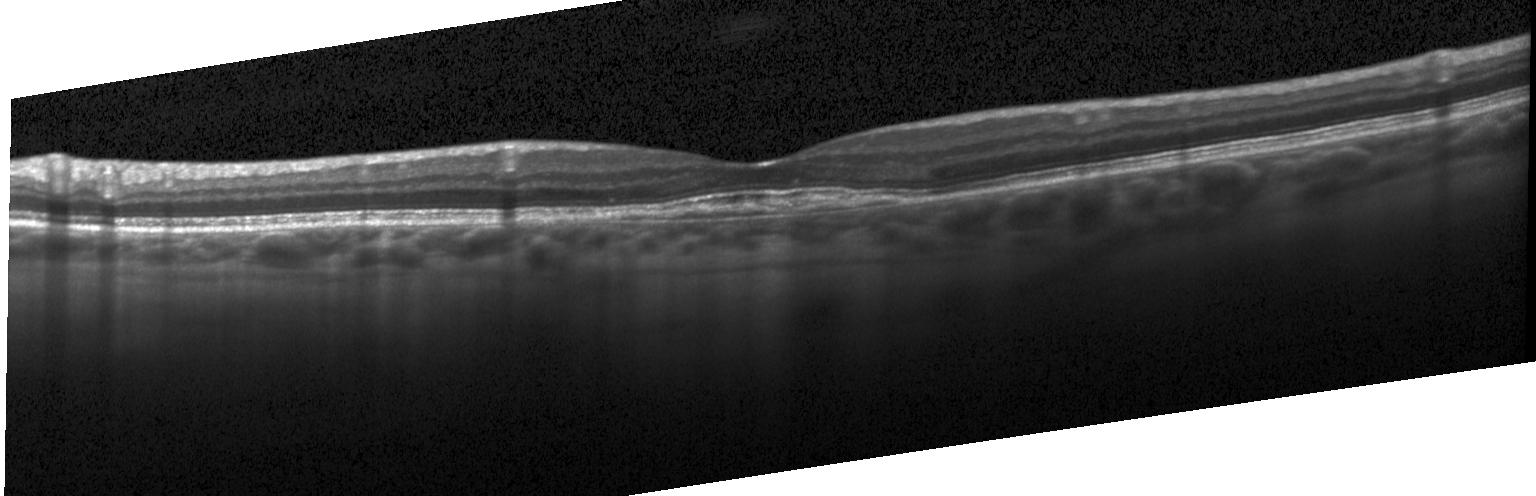 OCT line scan · centered on the fovea. Finding: a choroidal neovascular membrane.